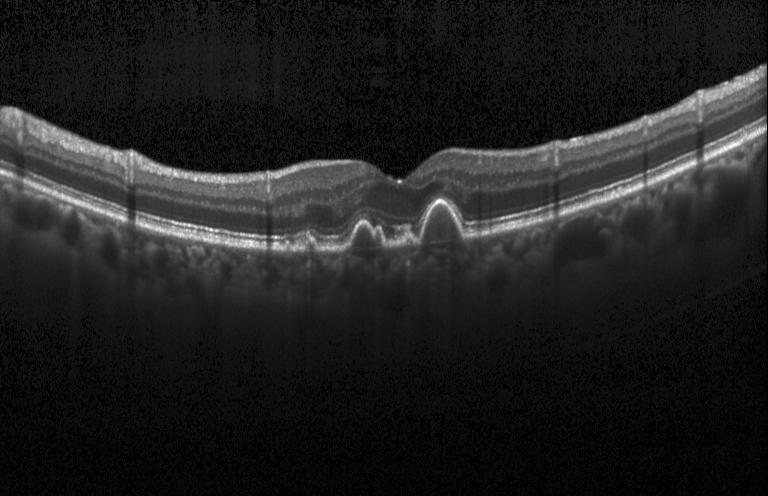 Diagnosis: sub-RPE drusenoid deposits.